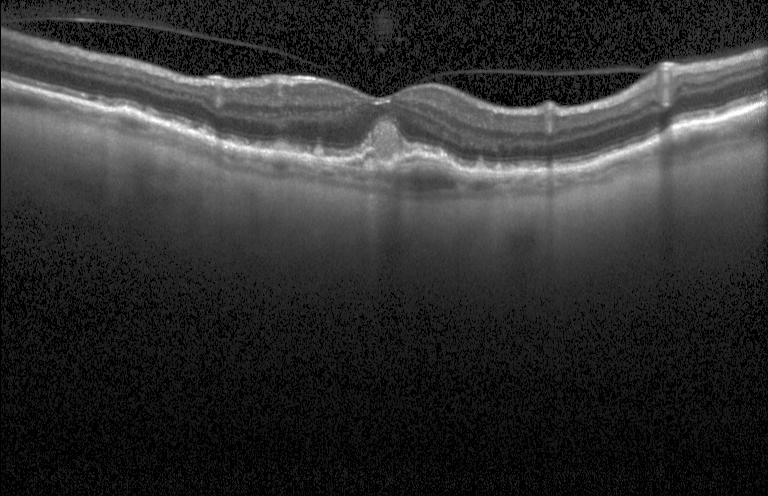 Spectral-domain OCT B-scan: choroidal neovascularization.